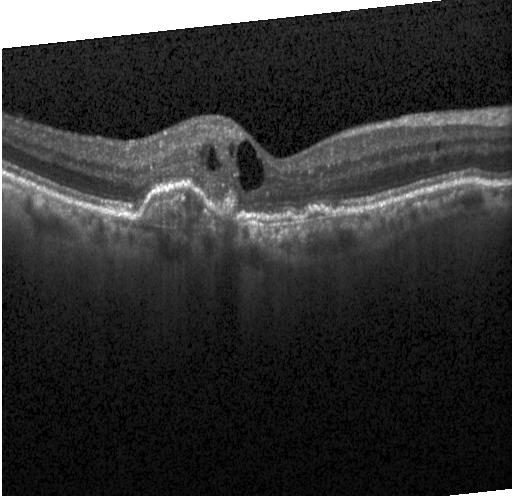 SD-OCT · OCT line scan · through the macula
This B-scan demonstrates a choroidal neovascular membrane.